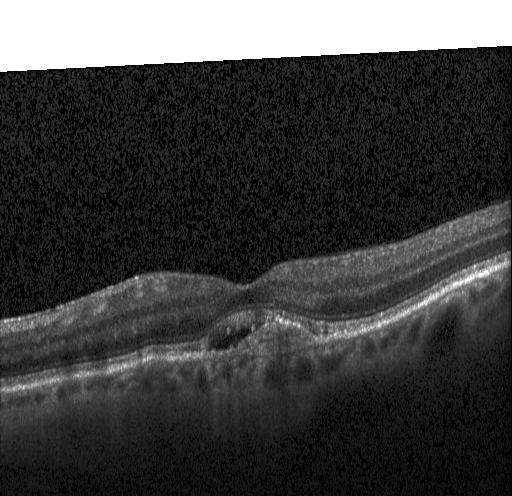

Retinal OCT B-scan
Assessment: a choroidal neovascular membrane.